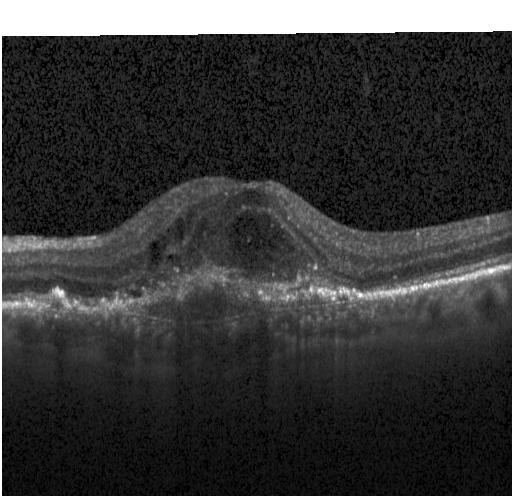 Spectral-domain OCT; optical coherence tomography scan
Finding: a choroidal neovascular membrane.